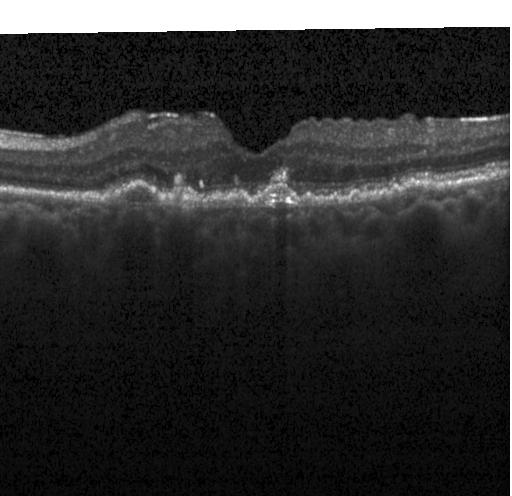
Optical coherence tomography B-scan. Spectral-domain OCT
OCT finding: CNV.